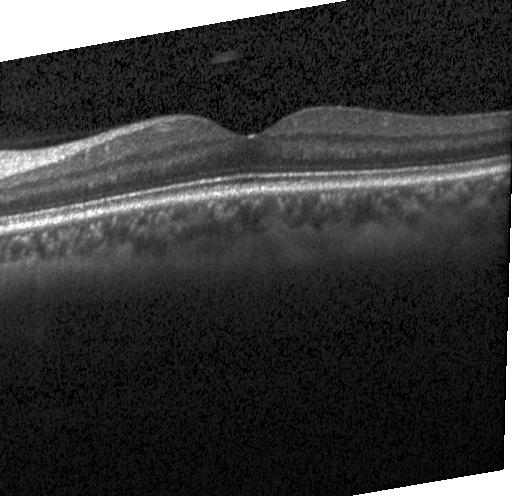
SD-OCT · optical coherence tomography scan.
Finding: no choroidal neovascularization, diabetic macular edema, or drusen.